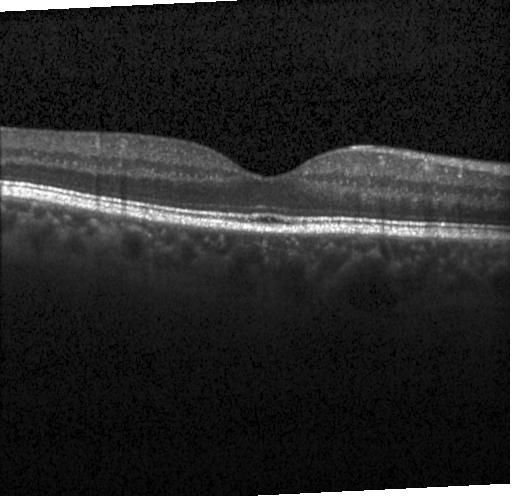

Fovea-centered, optical coherence tomography B-scan, acquired on a Heidelberg Spectralis.
Finding: no evidence of choroidal neovascularization, diabetic macular edema, or drusen.